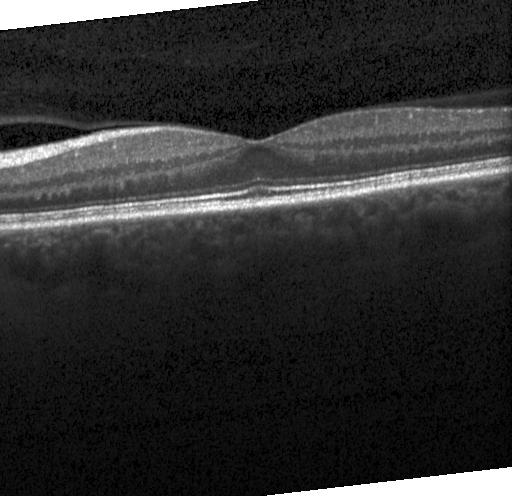 Finding: neither choroidal neovascularization, diabetic macular edema, nor drusen.